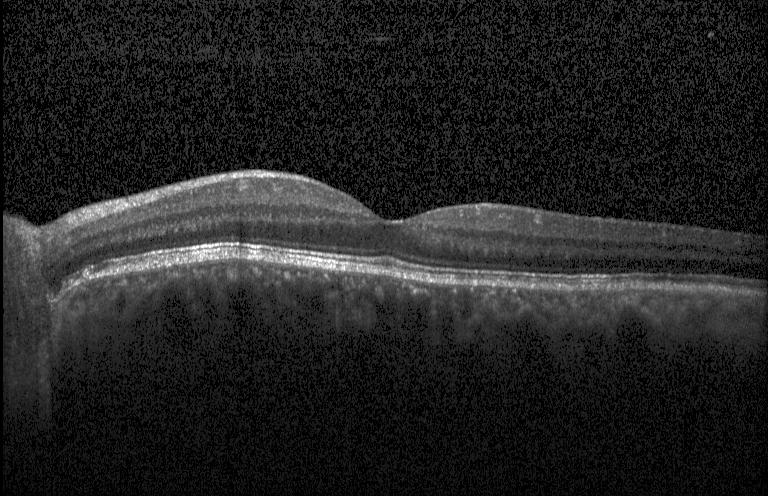

Finding: neither CNV, DME, nor drusen.